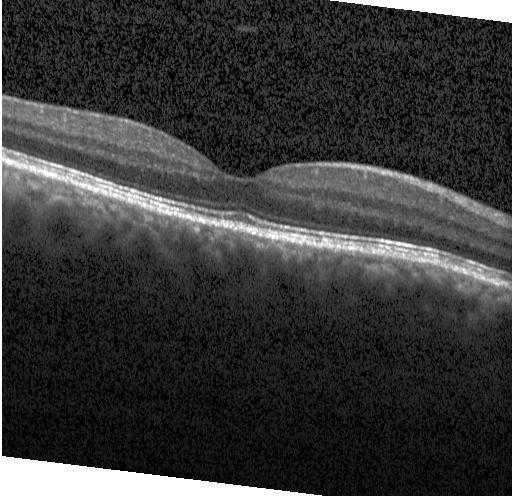 Impression: neither choroidal neovascularization, diabetic macular edema, nor drusen.